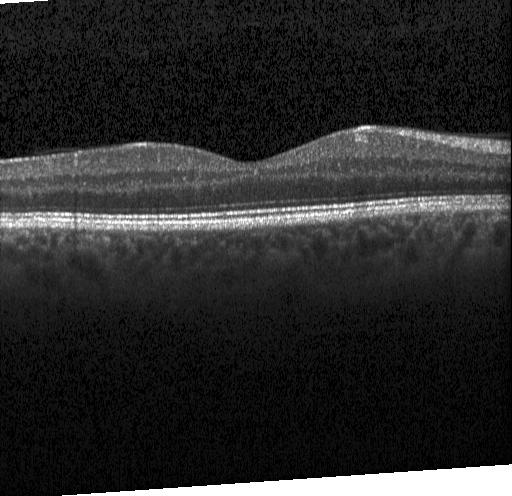

Diagnosis: no choroidal neovascularization, no diabetic macular edema, and no drusen.